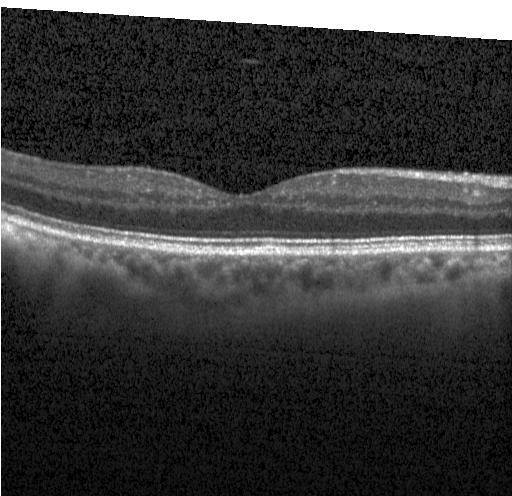 Impression: no evidence of choroidal neovascularization, diabetic macular edema, or drusen.